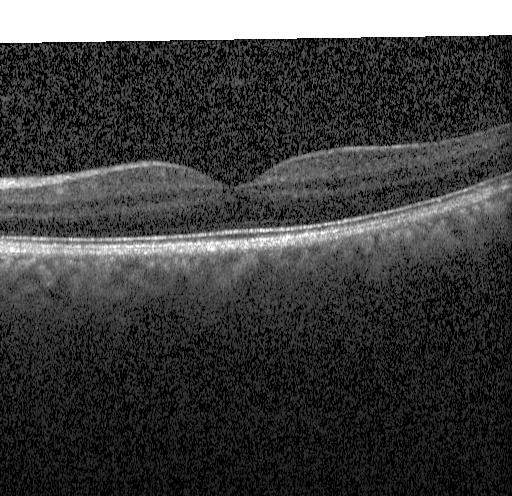 No choroidal neovascularization, diabetic macular edema, or drusen.